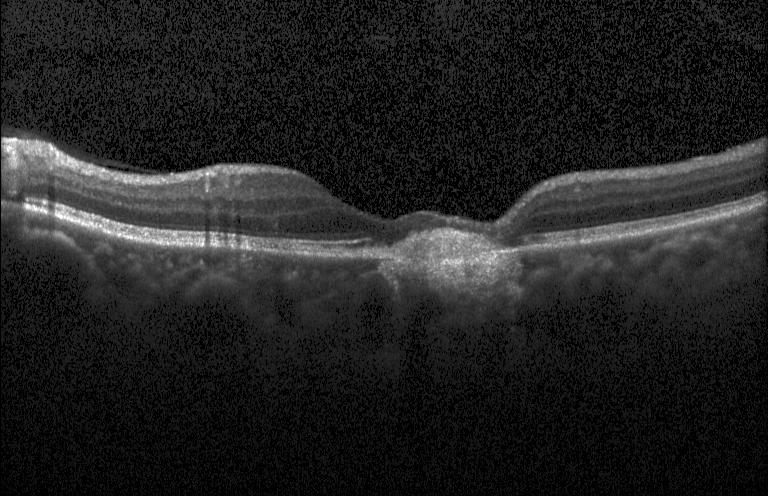

Spectral-domain OCT; horizontal scan through the fovea; Heidelberg Spectralis; optical coherence tomography B-scan — This B-scan demonstrates a choroidal neovascular membrane.